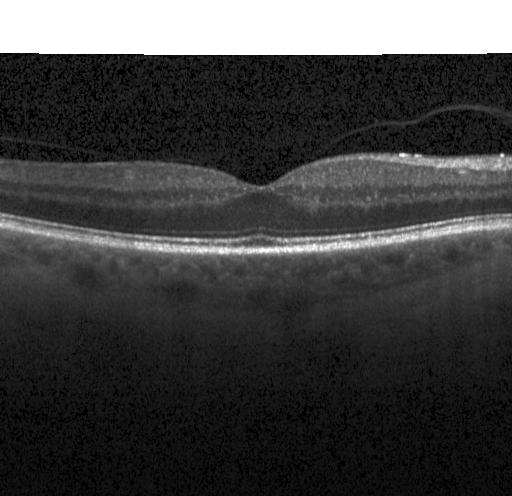

Fovea-centered, spectral-domain optical coherence tomography, acquired on a Heidelberg Spectralis, optical coherence tomography scan
Impression: no CNV, no DME, and no drusen.